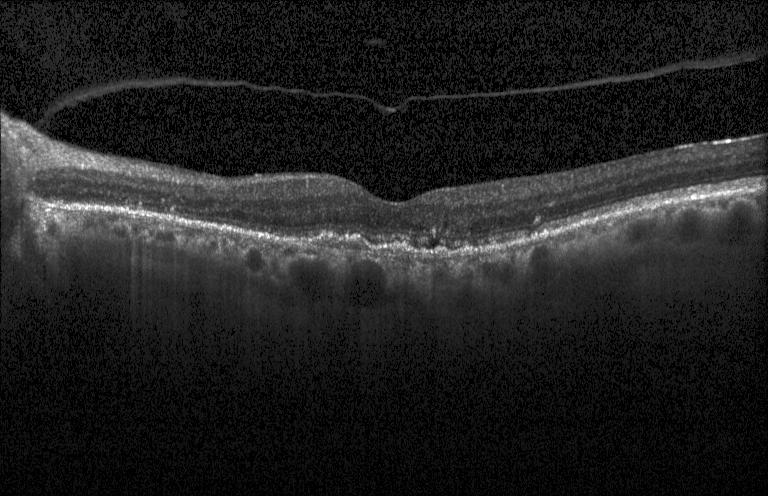

Finding: a choroidal neovascular membrane.